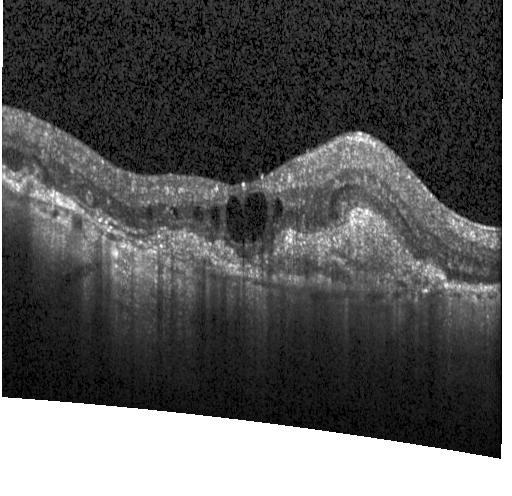
Optical coherence tomography B-scan — Macular OCT: a choroidal neovascular membrane.